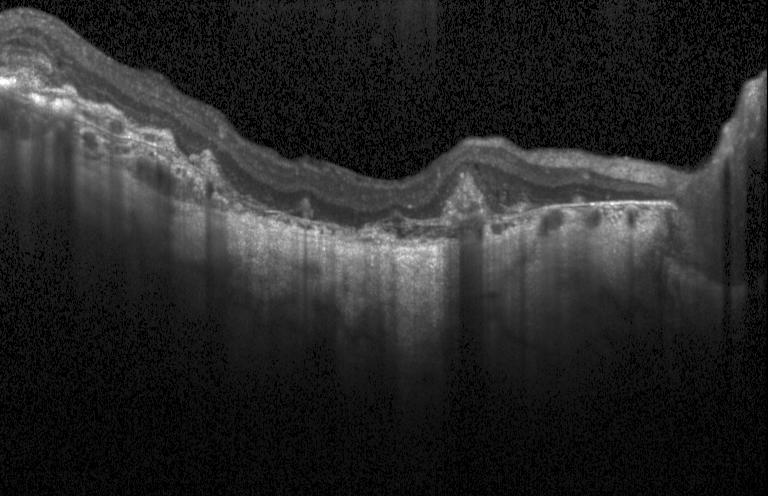

Dx: a choroidal neovascular membrane.